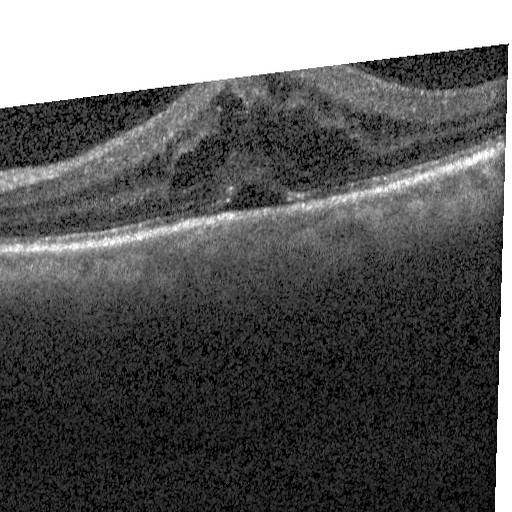 Instrument: Heidelberg Spectralis, OCT B-scan. The scan shows diabetic macular edema.